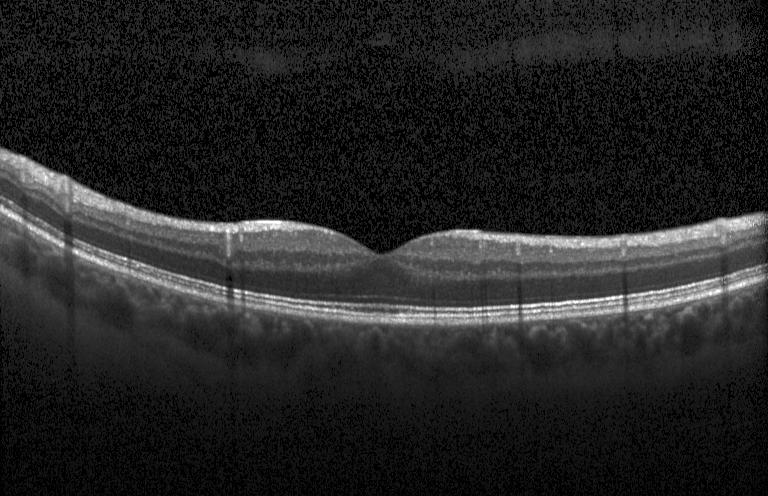 Heidelberg Spectralis OCT system, fovea-centered, optical coherence tomography scan
Finding: neither choroidal neovascularization, diabetic macular edema, nor drusen.